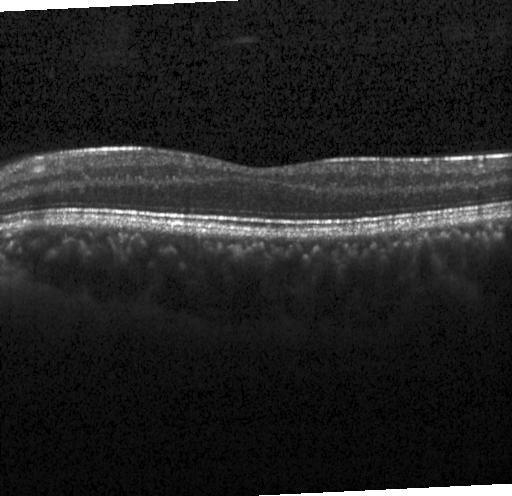
Impression: no choroidal neovascularization, no diabetic macular edema, and no drusen.